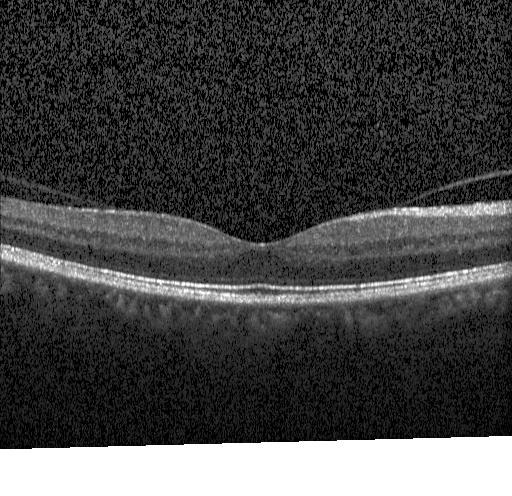

Spectral-domain OCT, optical coherence tomography B-scan, horizontal scan through the fovea.
Finding: no choroidal neovascularization, diabetic macular edema, or drusen.